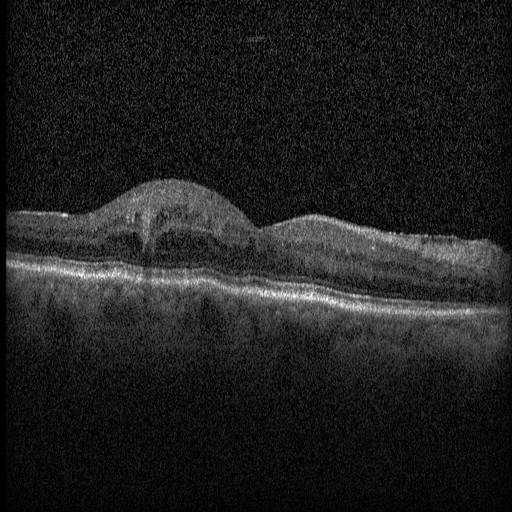 Macular OCT demonstrating diabetic macular edema.